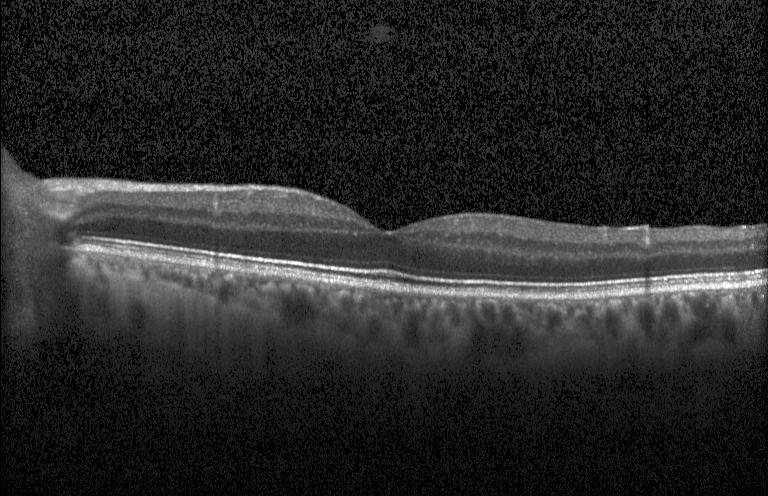
Optical coherence tomography B-scan. Spectral-domain optical coherence tomography. Macular scan. Heidelberg Spectralis.
Assessment: no choroidal neovascularization, diabetic macular edema, or drusen.